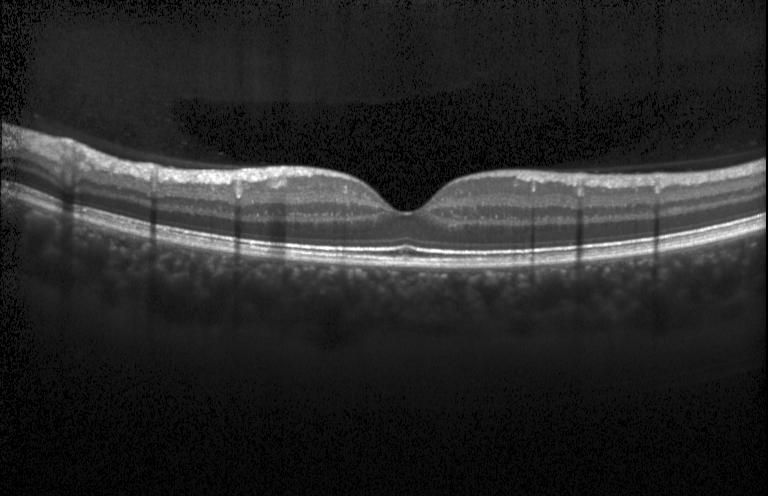 Acquired on a Heidelberg Spectralis, spectral-domain optical coherence tomography, optical coherence tomography scan.
Assessment: no CNV, DME, or drusen.